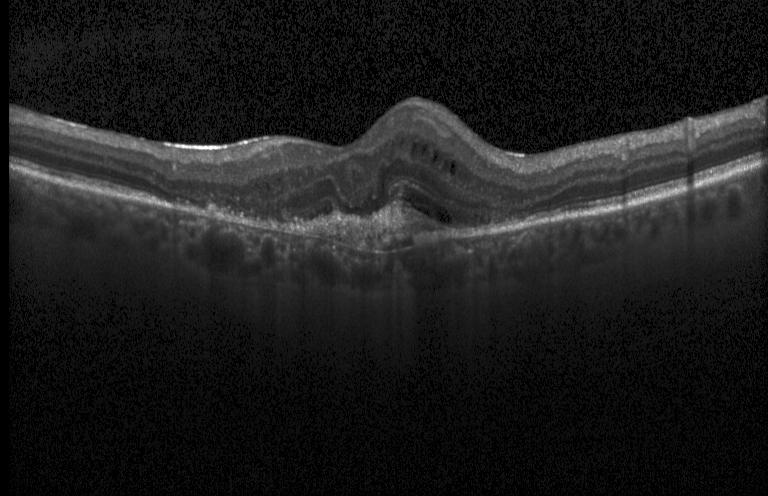 Macular scan · SD-OCT · OCT line scan
Impression: a choroidal neovascular membrane.